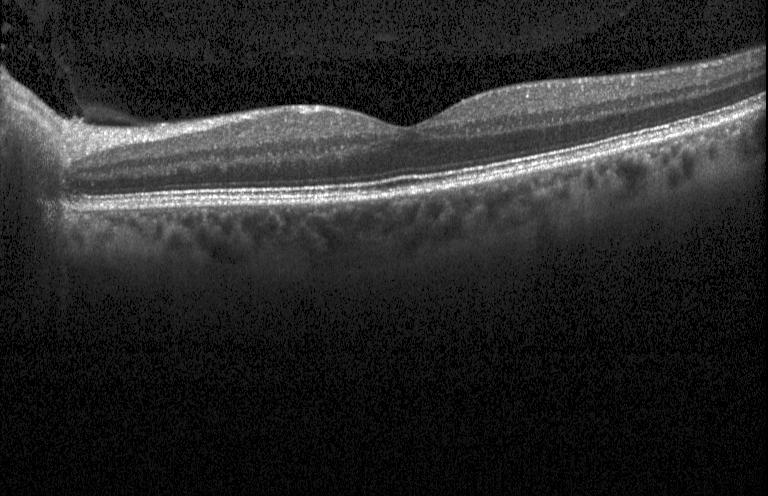 Optical coherence tomography B-scan; SD-OCT — Assessment: no CNV, no DME, and no drusen.